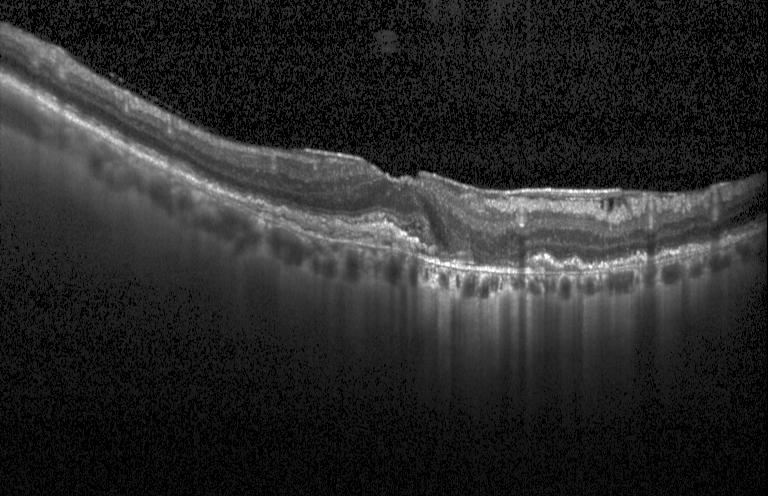
OCT line scan
Finding: a choroidal neovascular membrane.